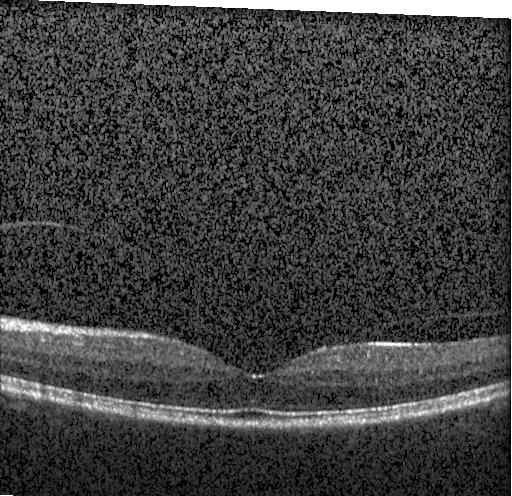
SD-OCT; optical coherence tomography B-scan — No choroidal neovascularization, no diabetic macular edema, and no drusen.